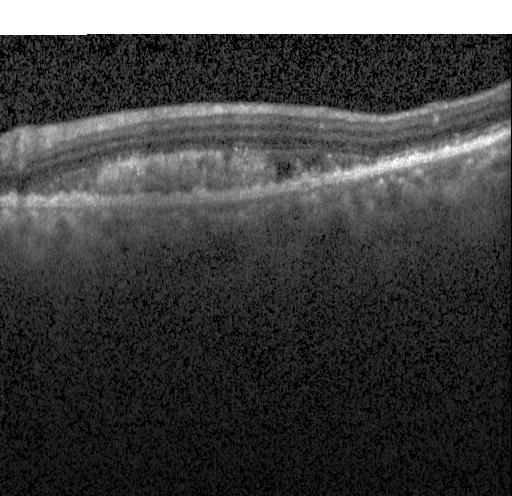
Retinal OCT B-scan; spectral-domain OCT; Heidelberg Spectralis
Finding: a choroidal neovascular membrane.